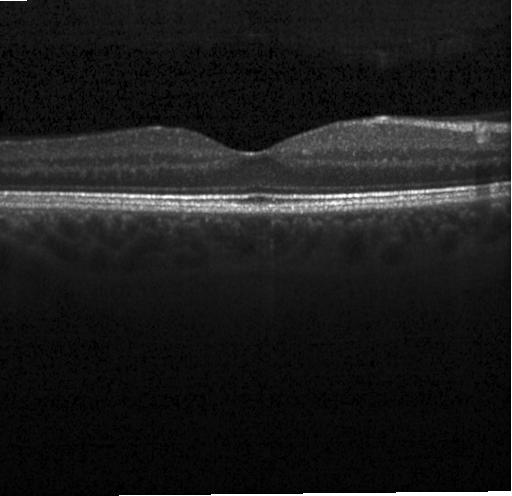

Retinal OCT cross-section.
Diagnosis: neither choroidal neovascularization, diabetic macular edema, nor drusen.